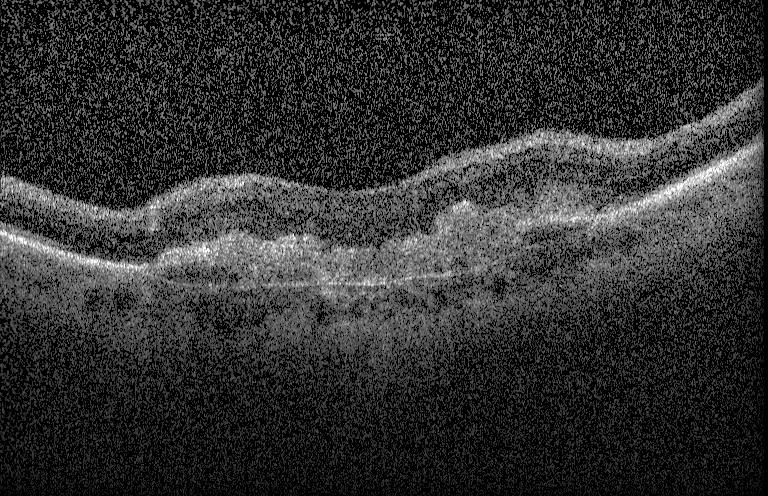 Optical coherence tomography scan; acquired on a Heidelberg Spectralis; spectral-domain optical coherence tomography
Impression: a choroidal neovascular membrane.